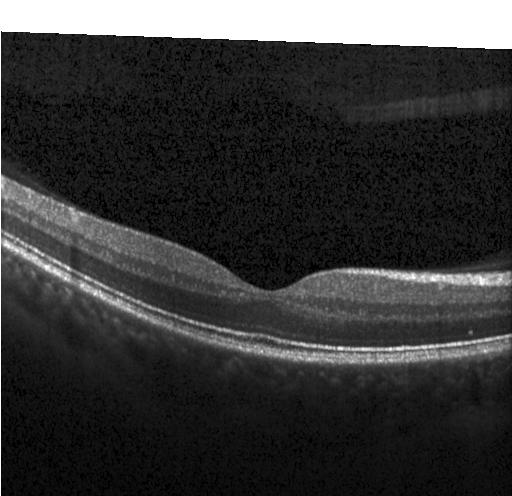 Heidelberg Spectralis OCT system, retinal OCT cross-section, centered on the fovea, SD-OCT. Diagnosis: no evidence of choroidal neovascularization, diabetic macular edema, or drusen.